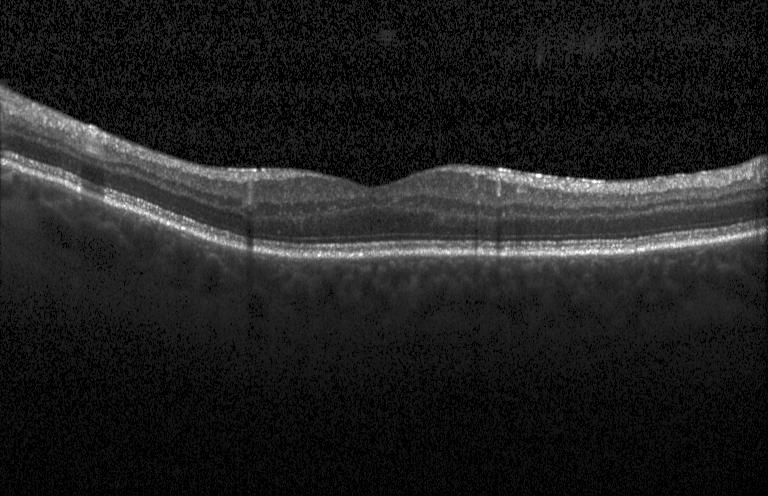 Centered on the fovea; spectral-domain OCT; acquired on a Heidelberg Spectralis; optical coherence tomography scan. Diagnosis: neither CNV, DME, nor drusen.